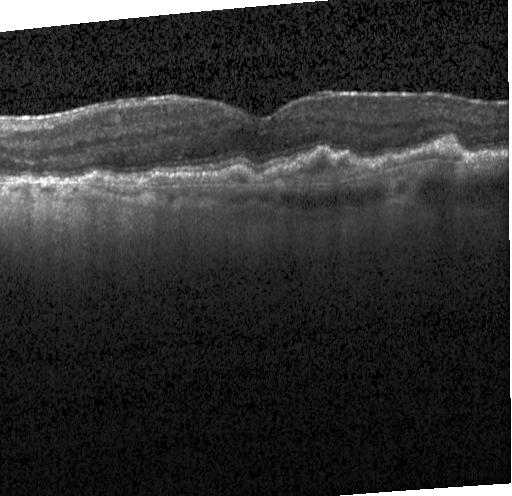 Spectral-domain OCT. Horizontal scan through the fovea. OCT B-scan. Instrument: Heidelberg Spectralis. Dx: choroidal neovascularization.